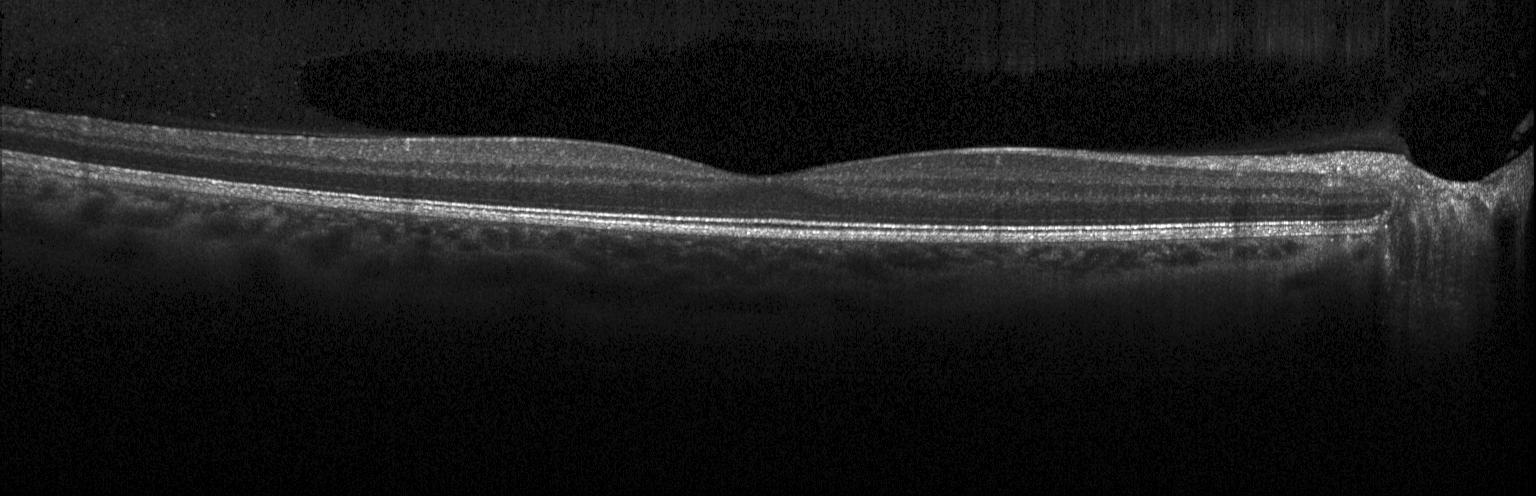

Assessment: neither choroidal neovascularization, diabetic macular edema, nor drusen.